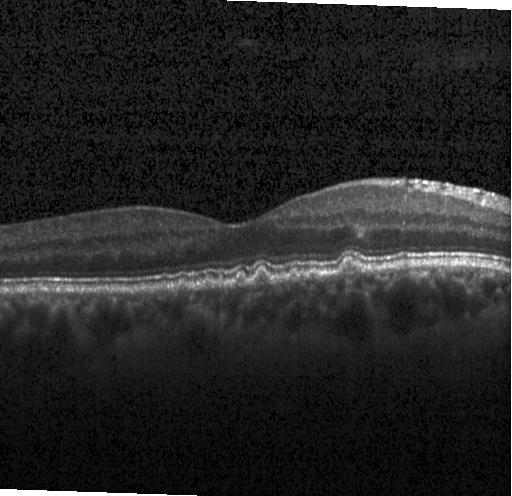

Finding: drusen.